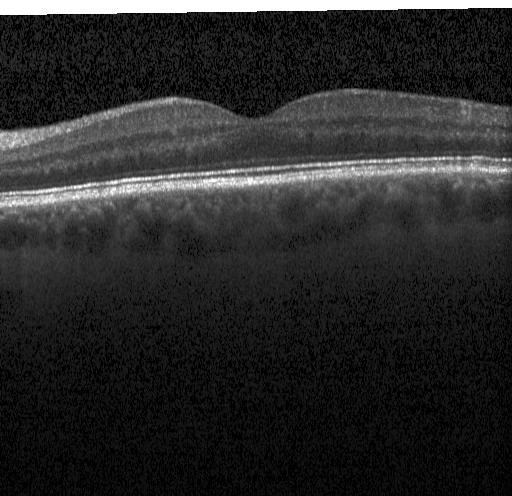 Retinal OCT B-scan, spectral-domain optical coherence tomography.
Macular OCT: no choroidal neovascularization, no diabetic macular edema, and no drusen.